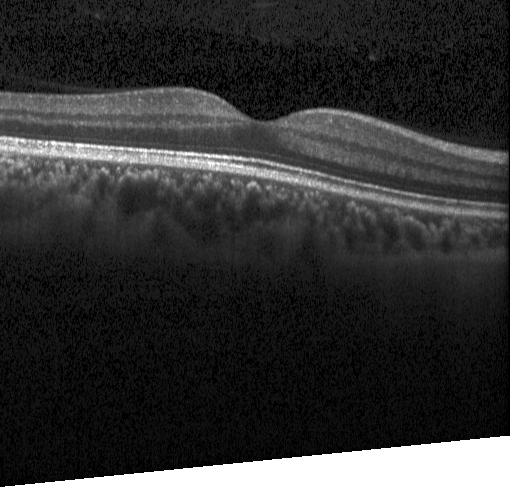
Dx: no choroidal neovascularization, diabetic macular edema, or drusen.